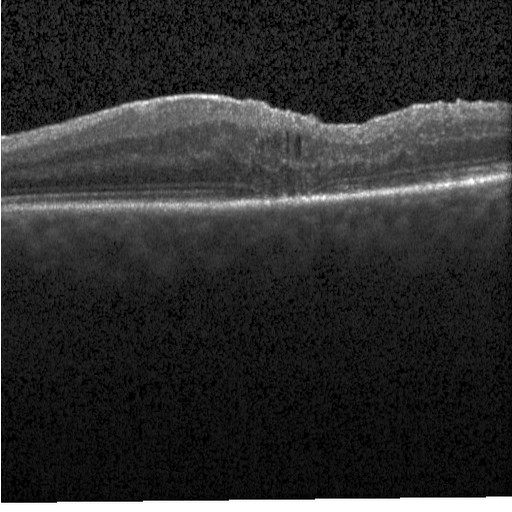
Finding: diabetic macular edema (DME).